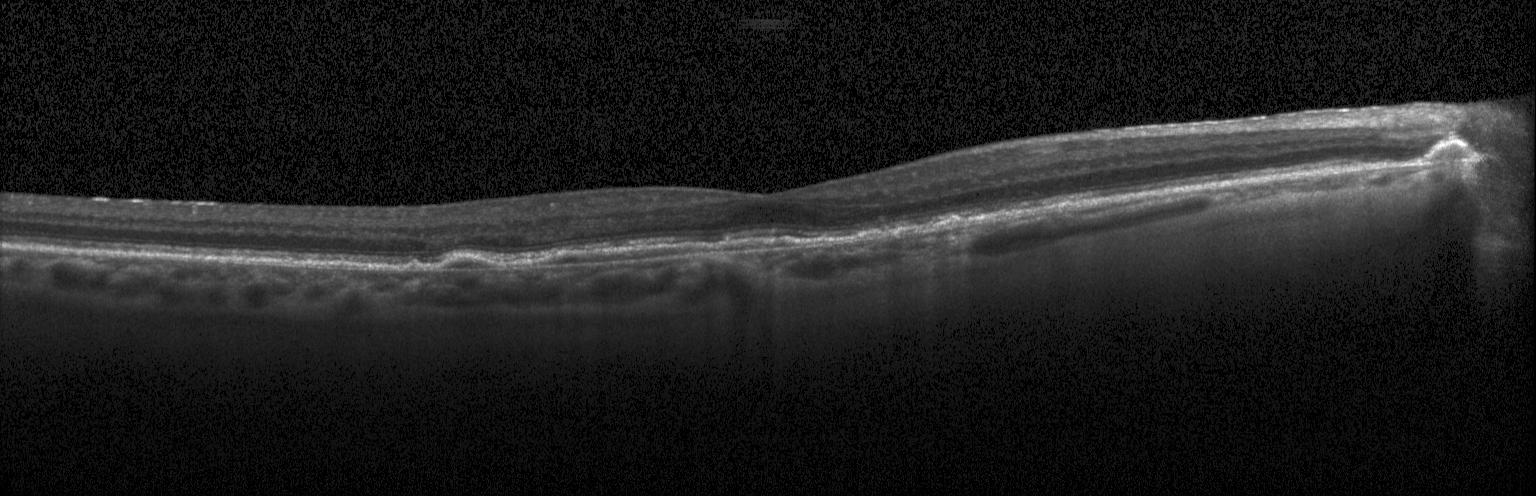
Centered on the fovea. Retinal OCT B-scan.
Assessment: CNV.